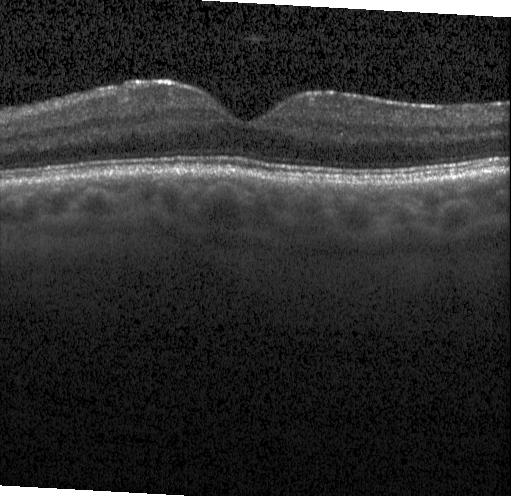 Heidelberg Spectralis OCT system; horizontal scan through the fovea; retinal OCT cross-section. Neither CNV, DME, nor drusen.